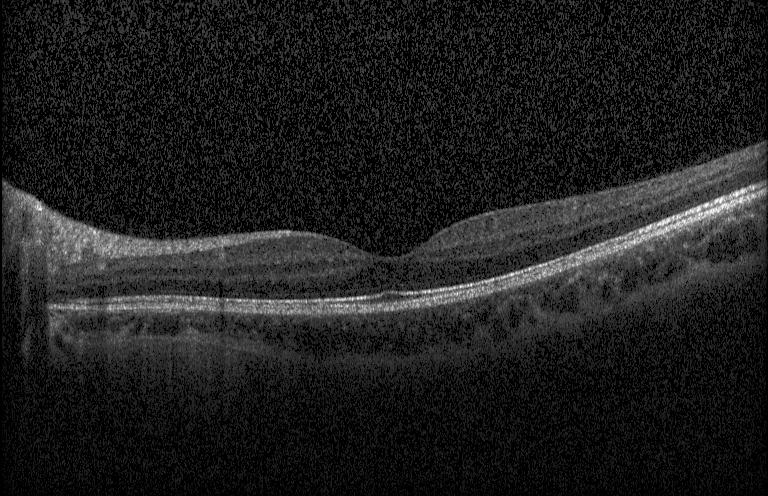

OCT B-scan. Finding: no evidence of CNV, DME, or drusen.